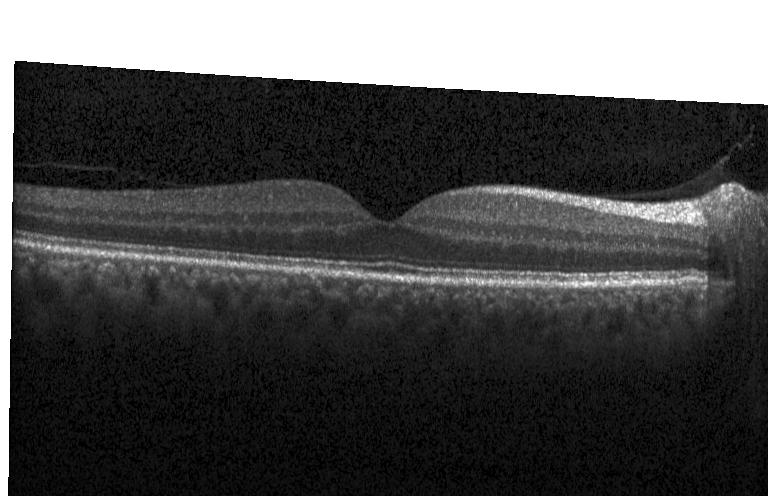

Retinal OCT cross-section.
Neither choroidal neovascularization, diabetic macular edema, nor drusen.